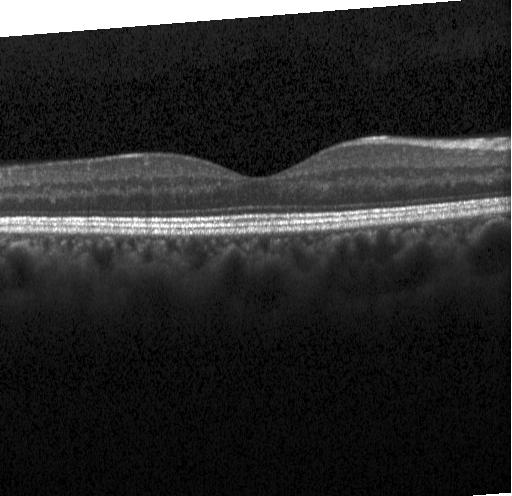

OCT B-scan showing neither choroidal neovascularization, diabetic macular edema, nor drusen.